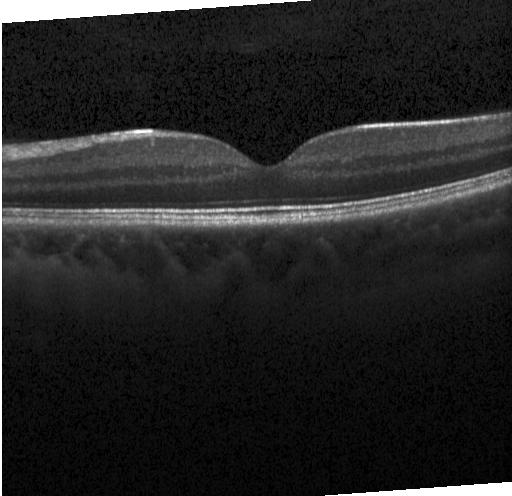

This B-scan demonstrates no evidence of choroidal neovascularization, diabetic macular edema, or drusen.